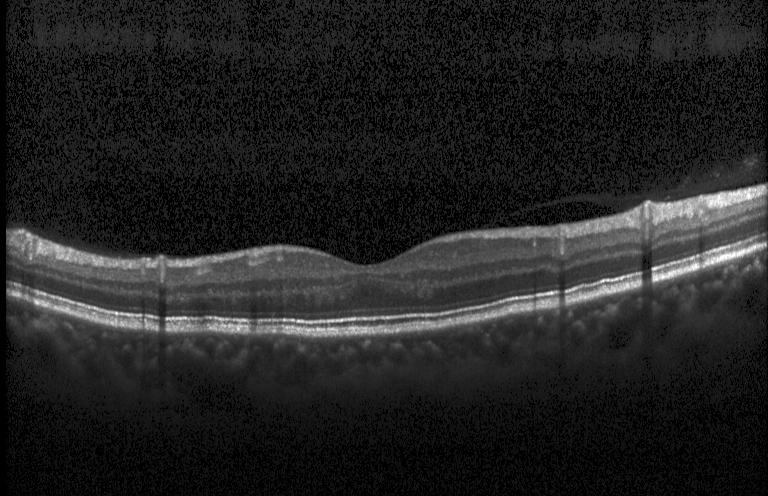

Spectral-domain OCT B-scan: no CNV, no DME, and no drusen.